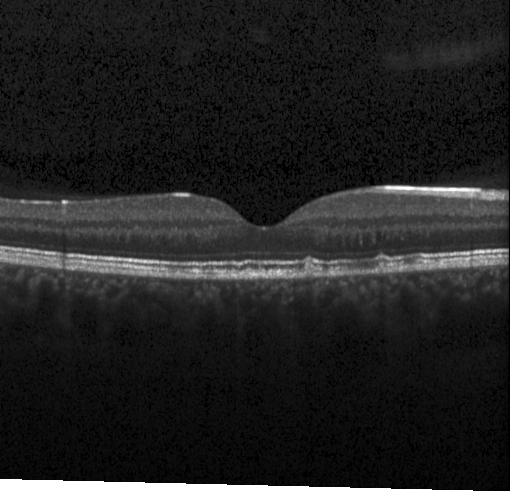

Macular OCT demonstrating sub-RPE drusenoid deposits.